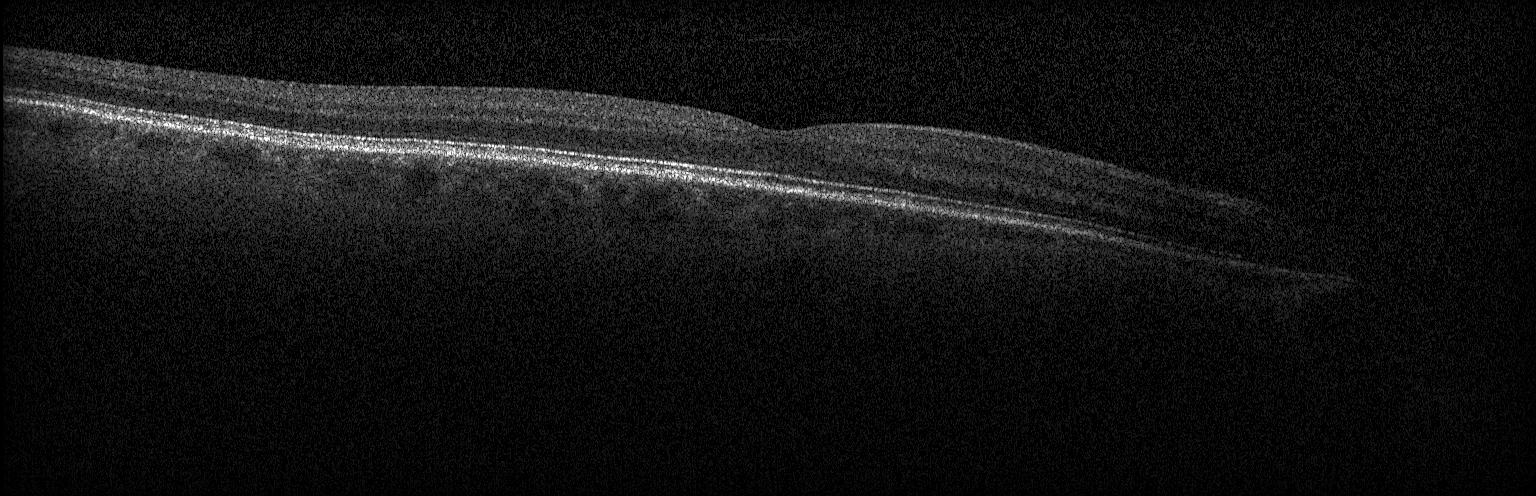

Macular OCT: no choroidal neovascularization, diabetic macular edema, or drusen.